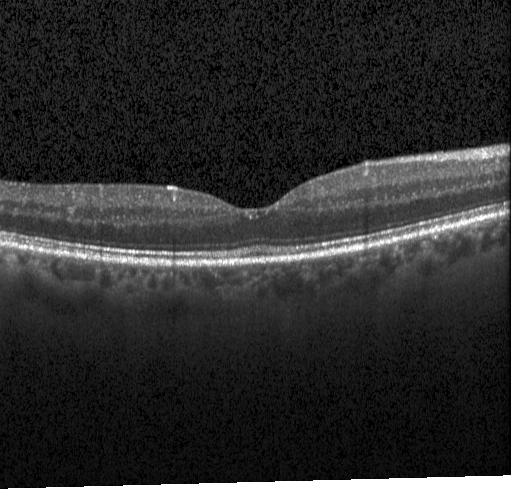

Macular scan. Retinal OCT B-scan
No choroidal neovascularization, no diabetic macular edema, and no drusen.